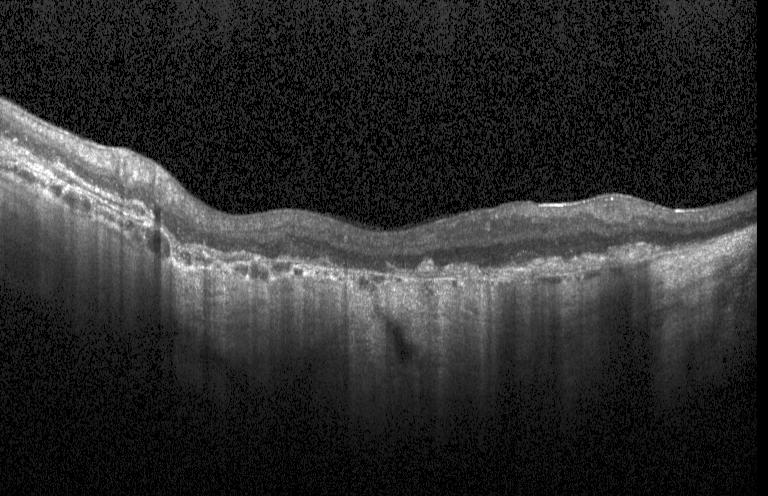

Impression: a choroidal neovascular membrane.